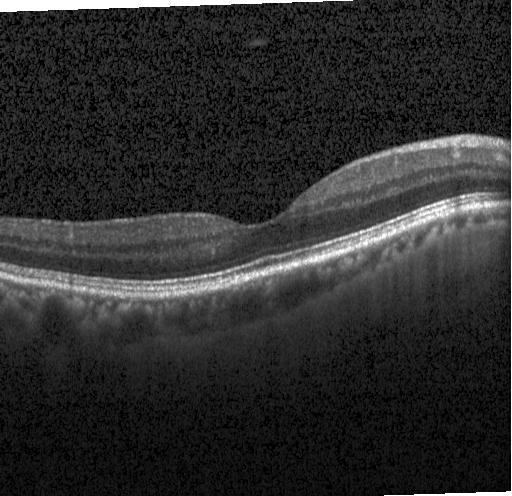

Acquired on a Heidelberg Spectralis; OCT line scan; horizontal scan through the fovea — The scan shows no choroidal neovascularization, diabetic macular edema, or drusen.